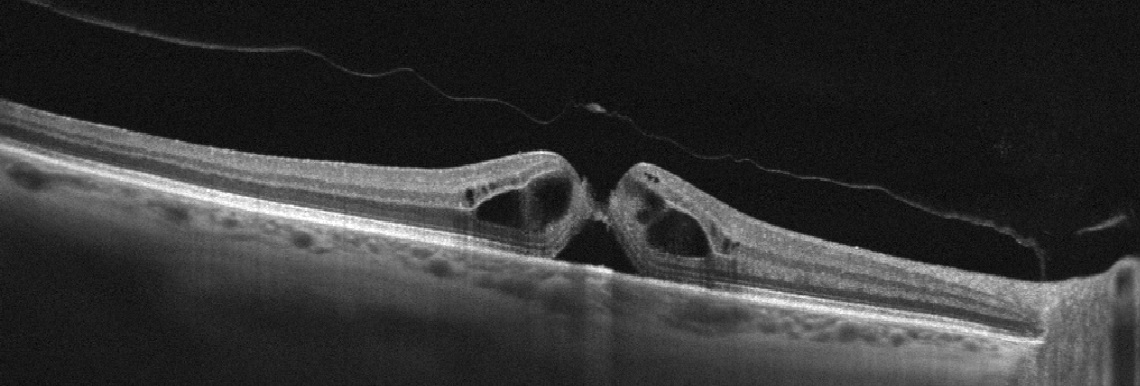

This B-scan demonstrates vitreomacular interface disease (VID).